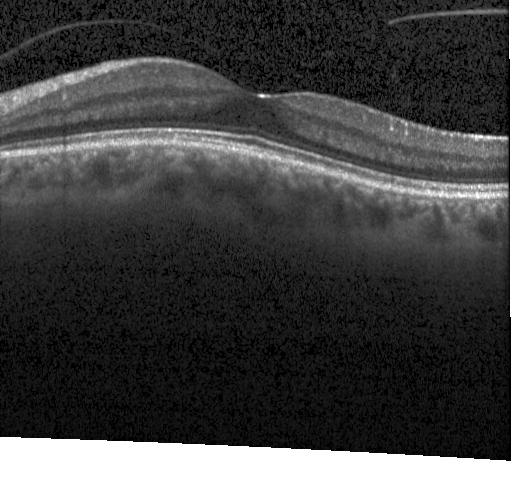
Macular scan, SD-OCT, instrument: Heidelberg Spectralis, retinal OCT cross-section. Finding: no choroidal neovascularization, no diabetic macular edema, and no drusen.